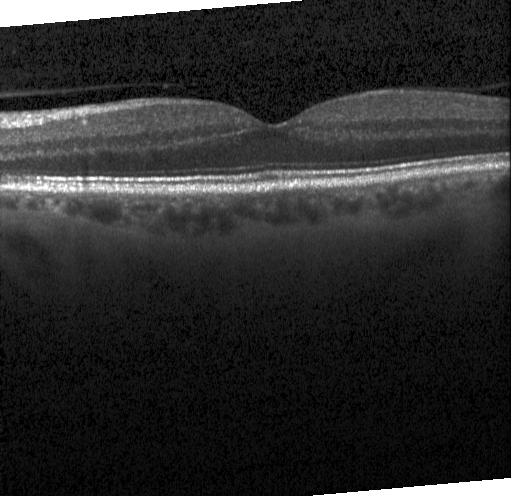
Dx: no choroidal neovascularization, no diabetic macular edema, and no drusen.